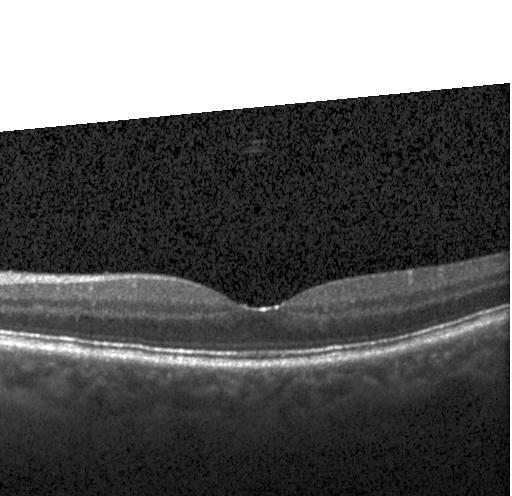 The scan shows no evidence of CNV, DME, or drusen.